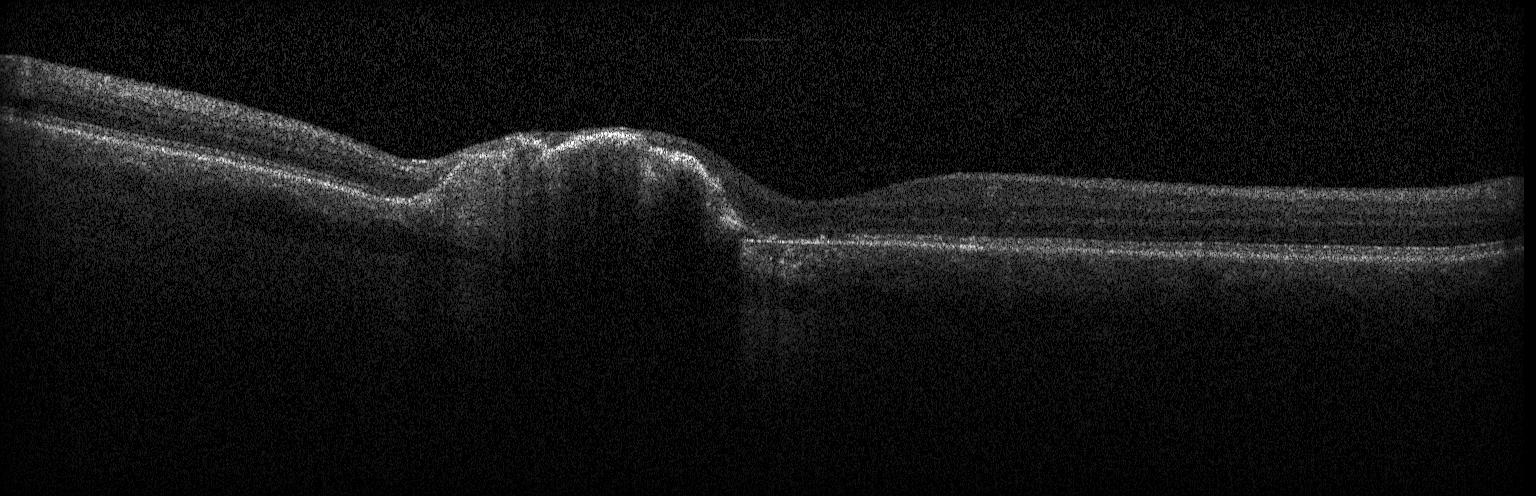 Retinal OCT B-scan — Dx: a choroidal neovascular membrane.